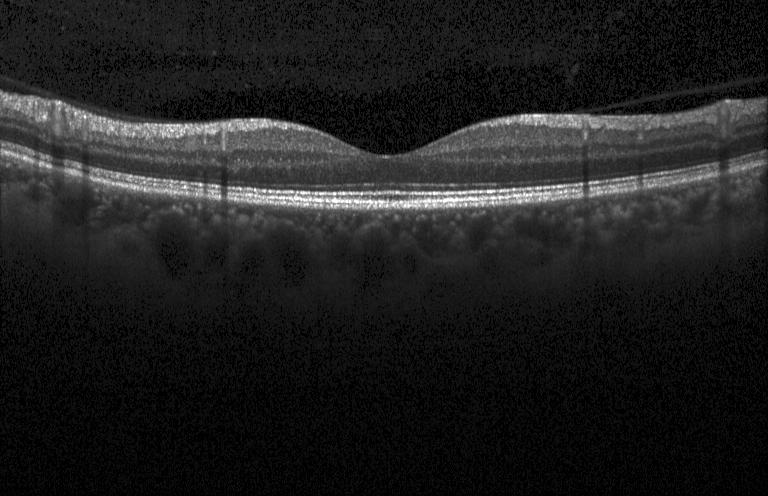 The scan shows no evidence of choroidal neovascularization, diabetic macular edema, or drusen.